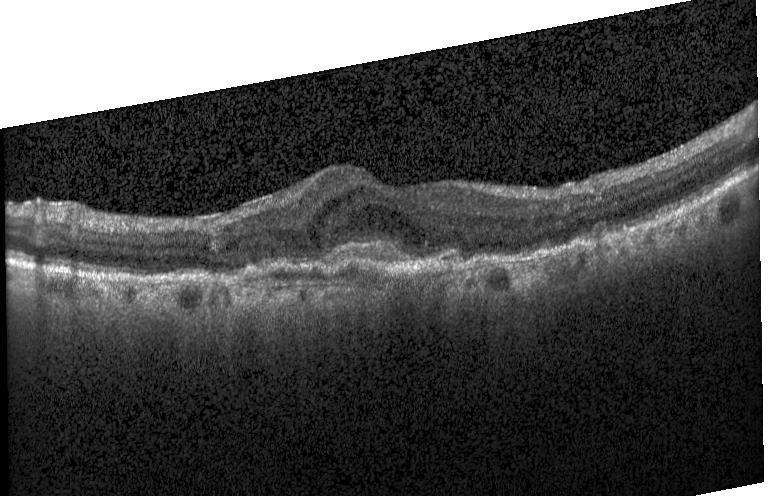

Through the macula. Heidelberg Spectralis. Optical coherence tomography scan.
The scan shows a choroidal neovascular membrane.